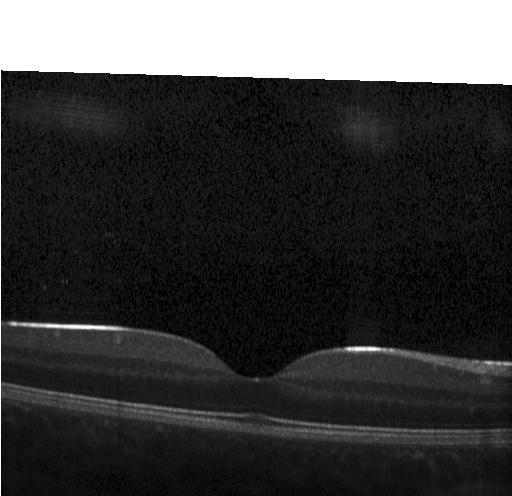

Retinal OCT cross-section, spectral-domain OCT, Heidelberg Spectralis OCT system, horizontal scan through the fovea. The scan shows no evidence of choroidal neovascularization, diabetic macular edema, or drusen.